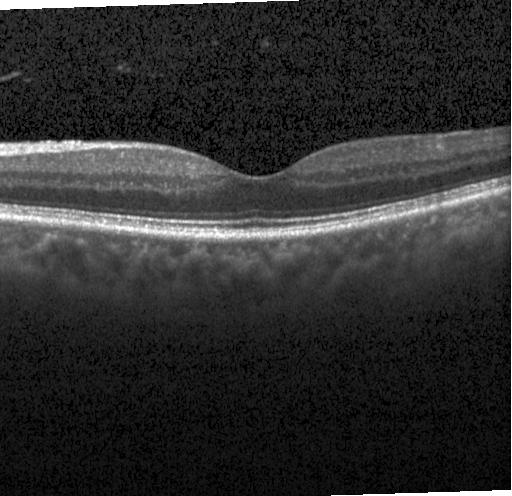
Optical coherence tomography B-scan — Neither CNV, DME, nor drusen.